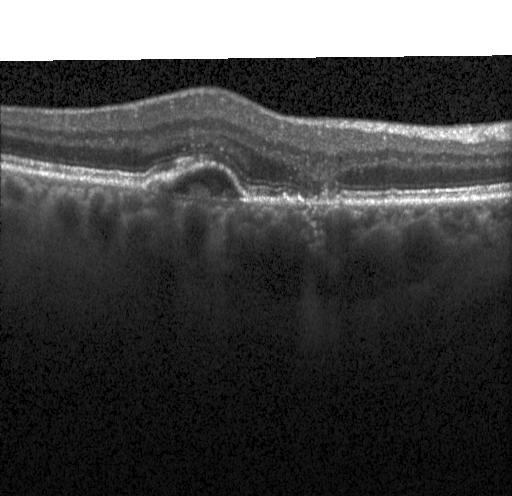 Dx: choroidal neovascularization.